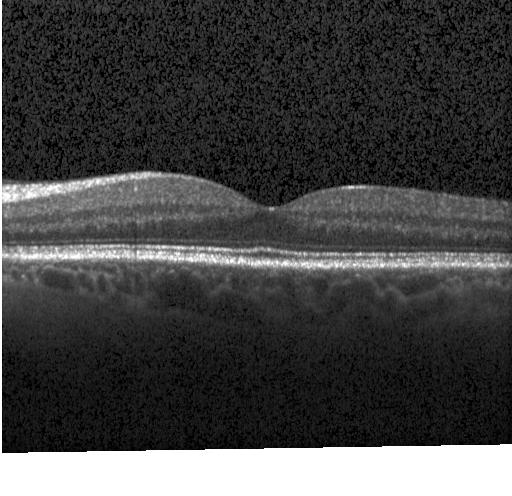

Optical coherence tomography scan
OCT finding: no evidence of choroidal neovascularization, diabetic macular edema, or drusen.